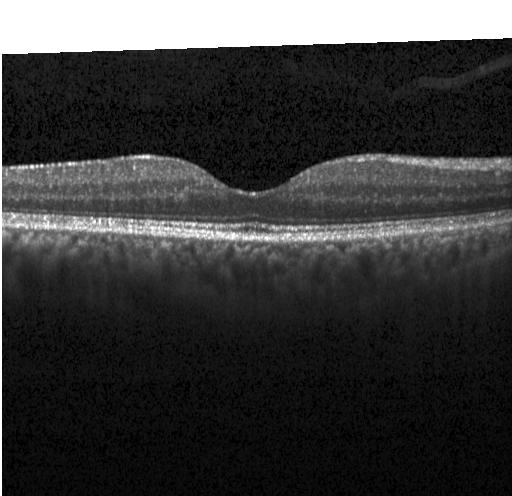
OCT line scan; spectral-domain optical coherence tomography.
No CNV, DME, or drusen.